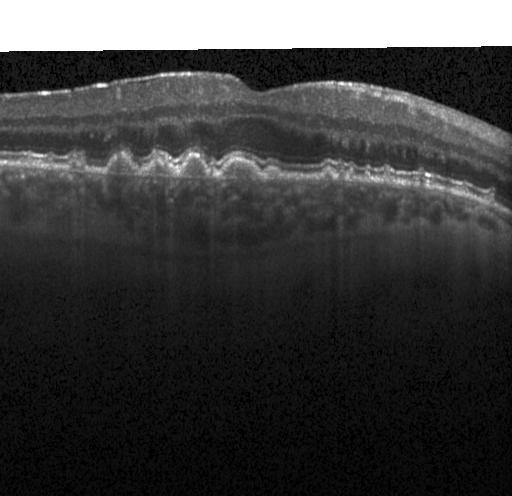 Heidelberg Spectralis OCT system. Macular scan. Optical coherence tomography B-scan. Spectral-domain optical coherence tomography
Assessment: CNV.